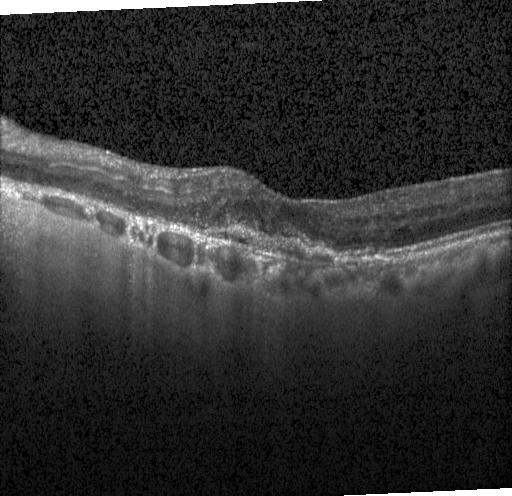 Retinal OCT B-scan; spectral-domain OCT; macular scan; acquired on a Heidelberg Spectralis.
CNV.